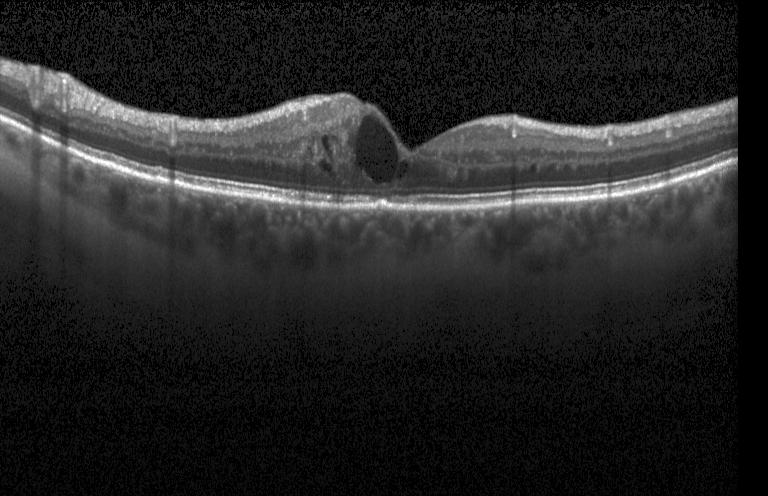

Macular OCT: diabetic macular edema (DME).